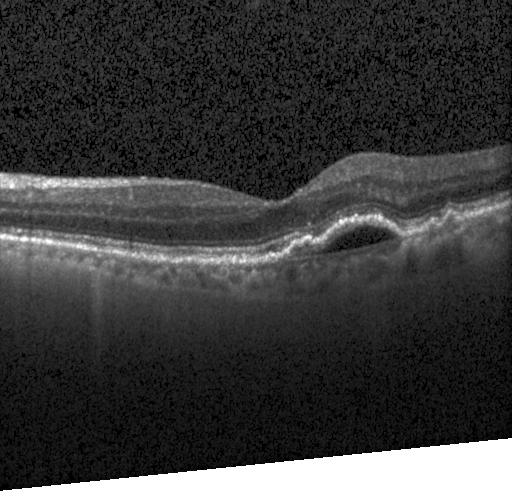

Optical coherence tomography scan. The scan shows CNV.